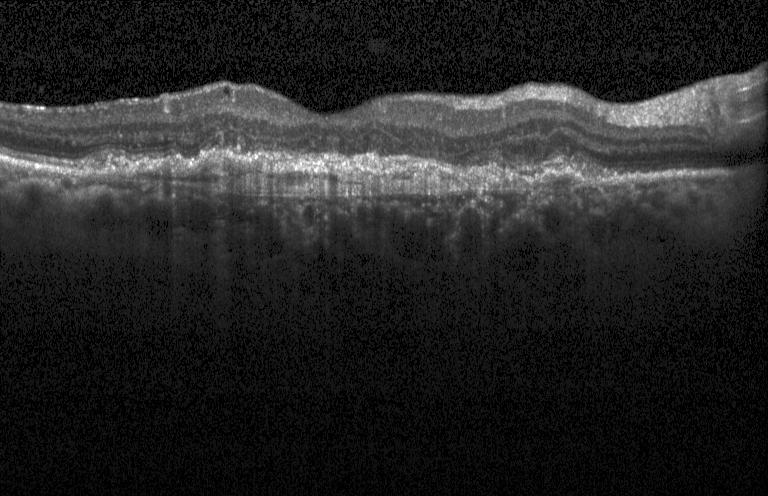

Acquired on a Heidelberg Spectralis, horizontal scan through the fovea, retinal OCT B-scan, SD-OCT. Finding: a choroidal neovascular membrane.